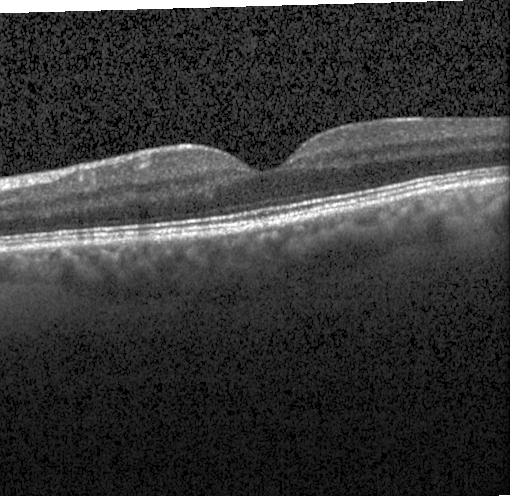

Centered on the fovea; optical coherence tomography scan.
OCT finding: neither choroidal neovascularization, diabetic macular edema, nor drusen.